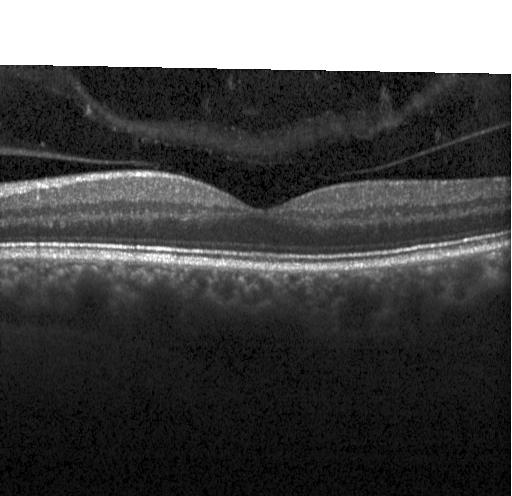

Horizontal scan through the fovea, OCT B-scan
Dx: no choroidal neovascularization, no diabetic macular edema, and no drusen.